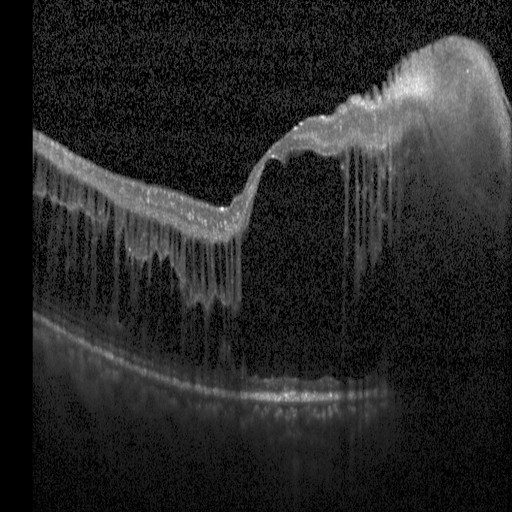

Acquired on a Heidelberg Spectralis. Optical coherence tomography B-scan.
The scan shows diabetic macular edema.